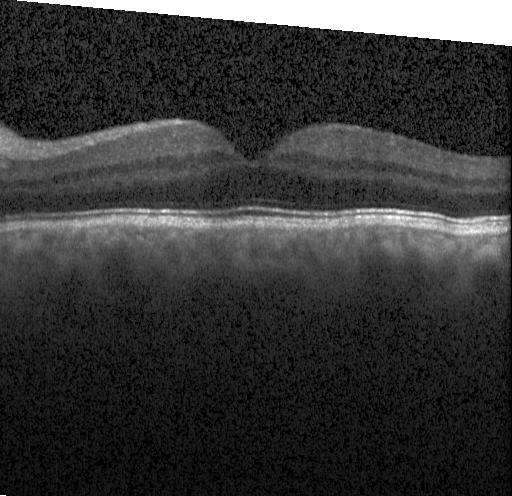
Spectral-domain OCT B-scan: no evidence of choroidal neovascularization, diabetic macular edema, or drusen.